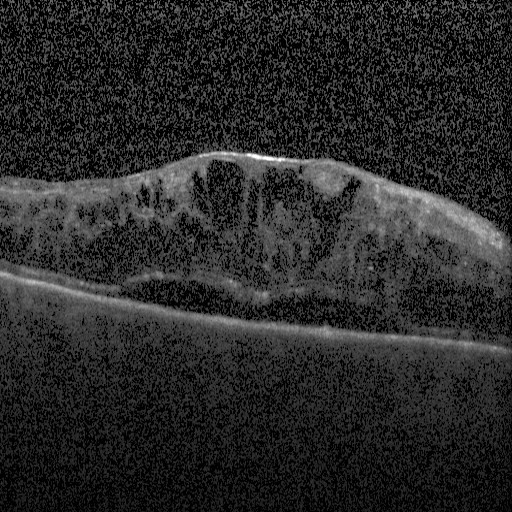
Heidelberg Spectralis OCT system · retinal OCT B-scan
Diagnosis: diabetic macular edema.